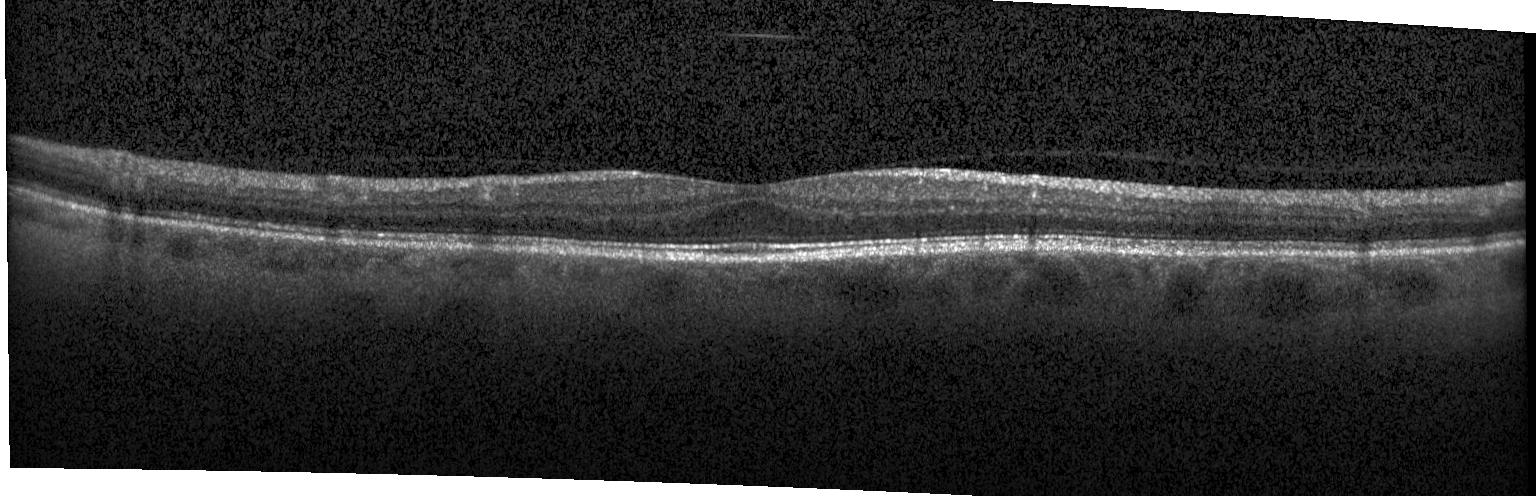 OCT scan showing no choroidal neovascularization, no diabetic macular edema, and no drusen.